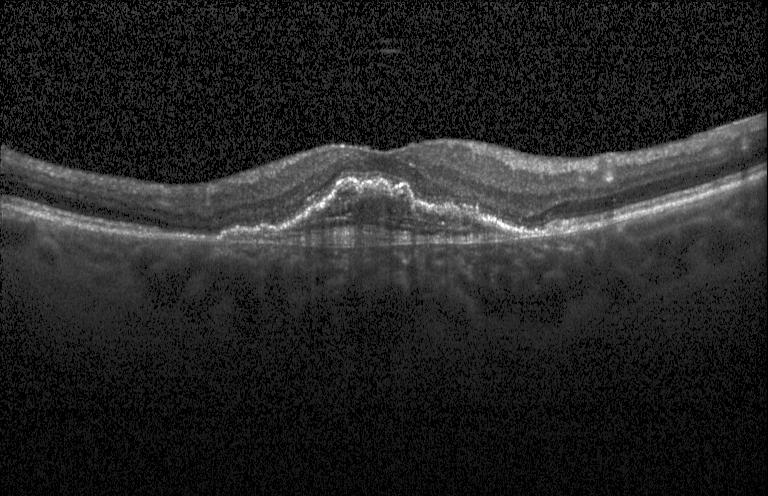 OCT line scan — Dx: a choroidal neovascular membrane.